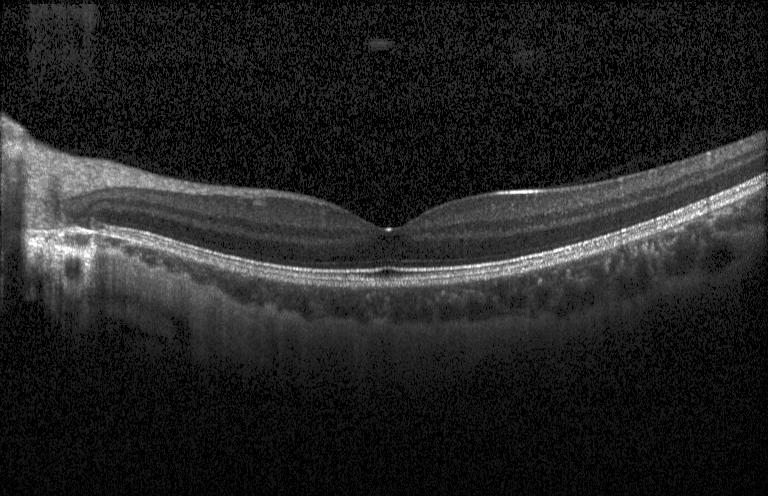
Instrument: Heidelberg Spectralis; centered on the fovea; OCT line scan — Impression: no choroidal neovascularization, no diabetic macular edema, and no drusen.